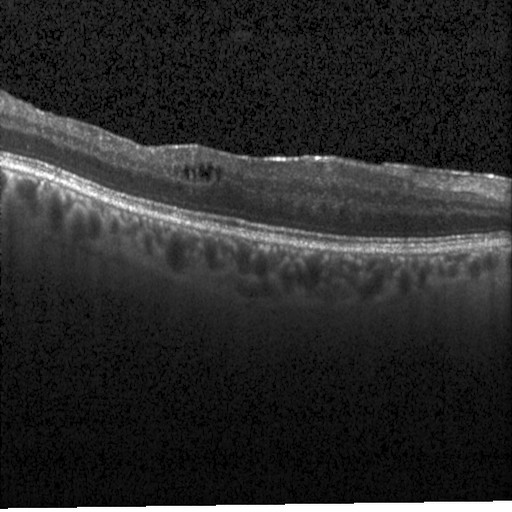
OCT B-scan — This B-scan demonstrates diabetic macular edema (DME).